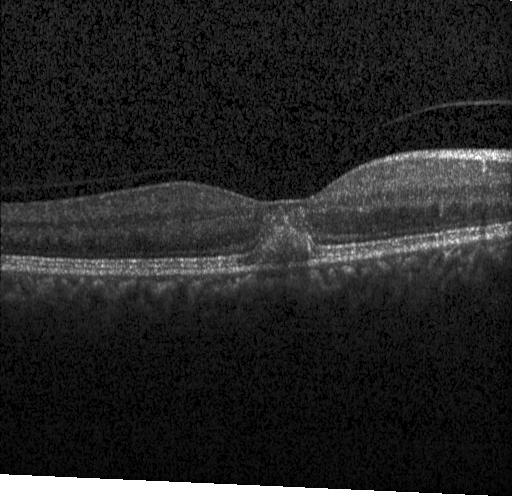 OCT B-scan showing a choroidal neovascular membrane.